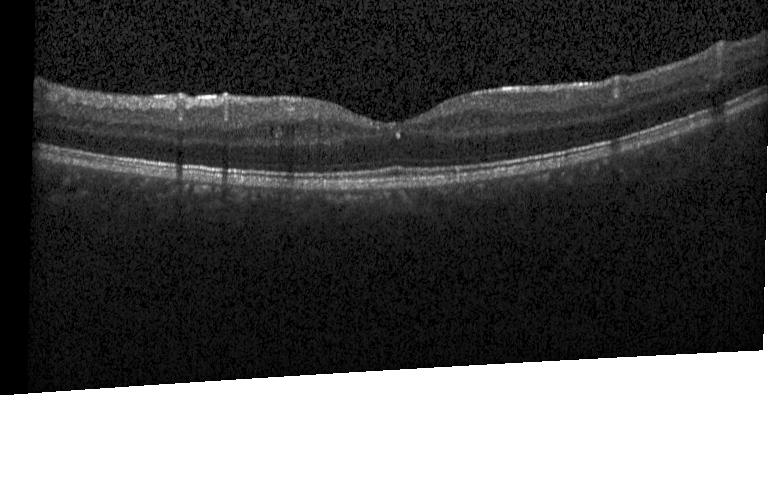 OCT line scan, SD-OCT. Dx: diabetic macular edema.